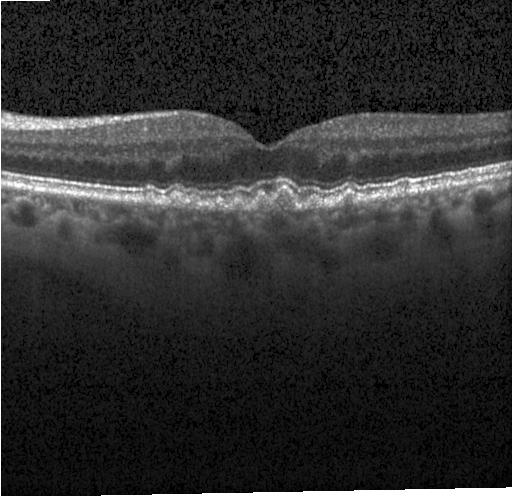 Through the macula, instrument: Heidelberg Spectralis, SD-OCT, optical coherence tomography scan — Drusen.